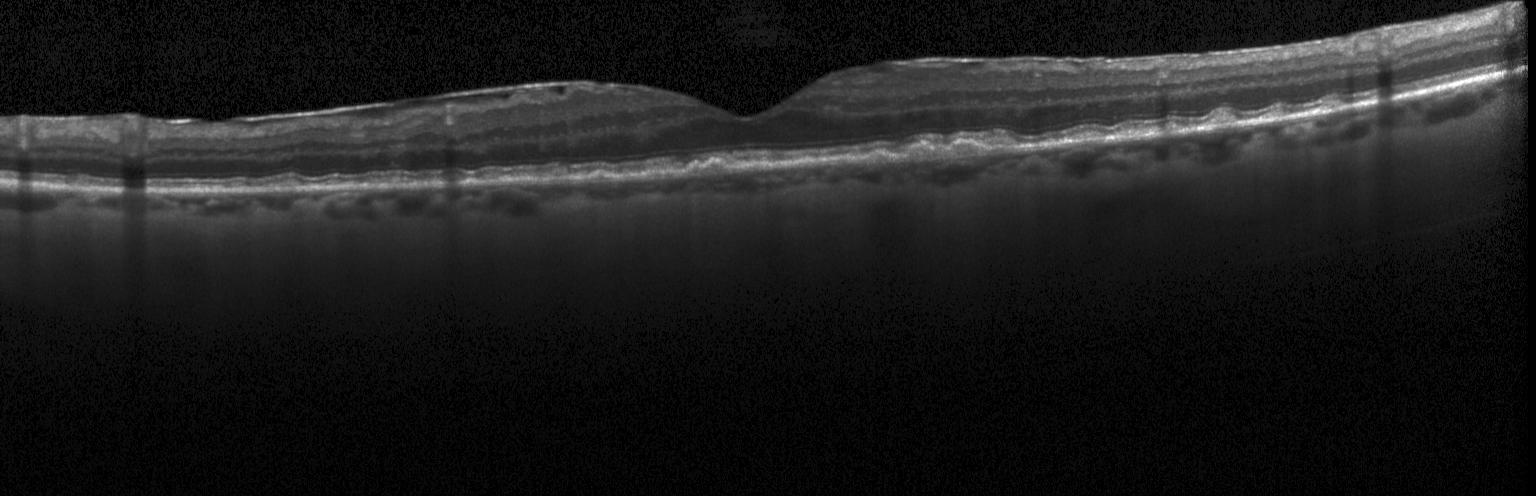 Macular scan. Retinal OCT B-scan. OCT finding: sub-RPE drusenoid deposits.